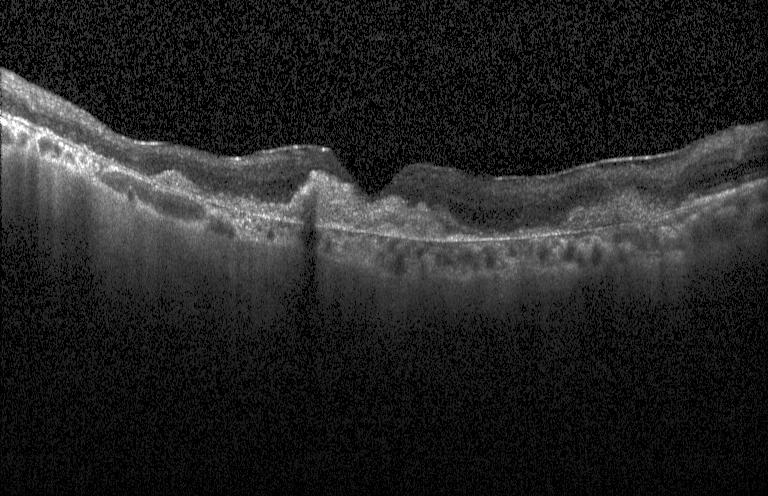

Diagnosis: a choroidal neovascular membrane.